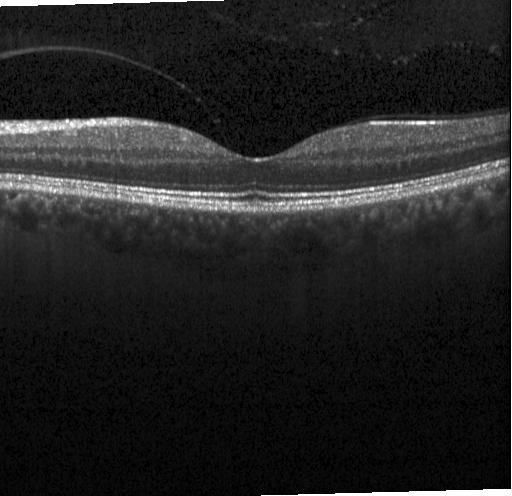

The scan shows no choroidal neovascularization, diabetic macular edema, or drusen.